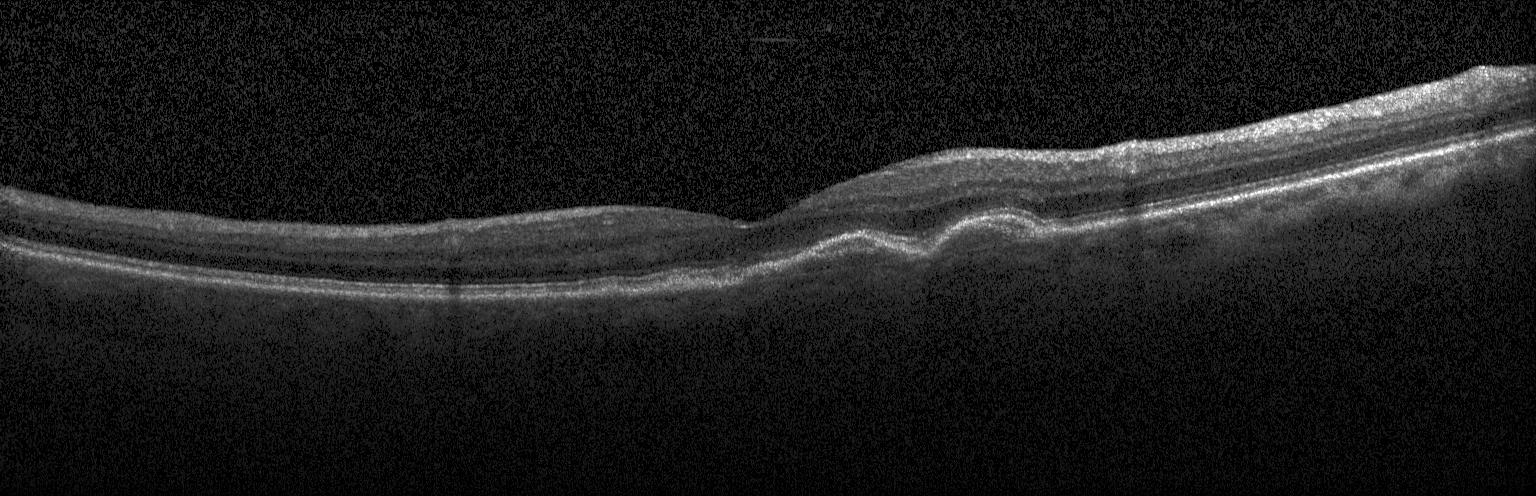 Retinal OCT cross-section. Heidelberg Spectralis OCT system. Spectral-domain OCT
Assessment: choroidal neovascularization (CNV).